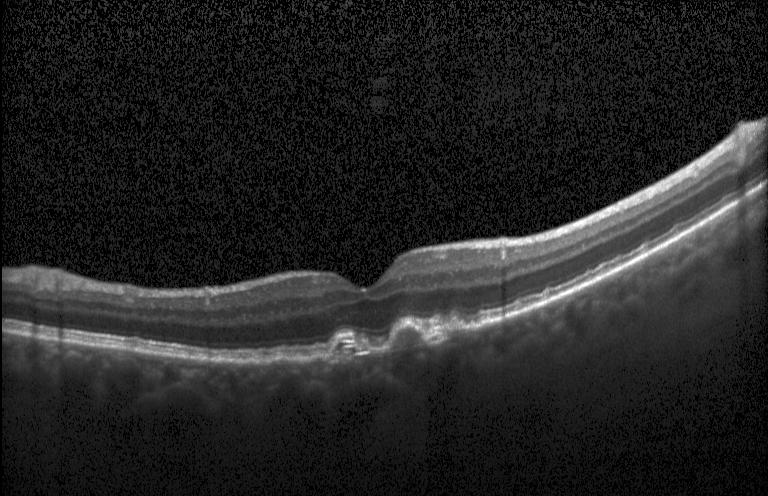

Heidelberg Spectralis; spectral-domain OCT; OCT line scan; centered on the fovea.
Diagnosis: a choroidal neovascular membrane.